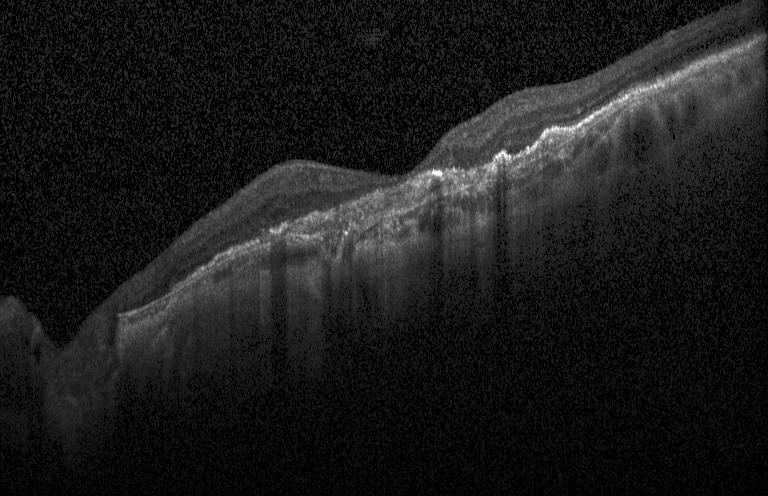

The scan shows a choroidal neovascular membrane.